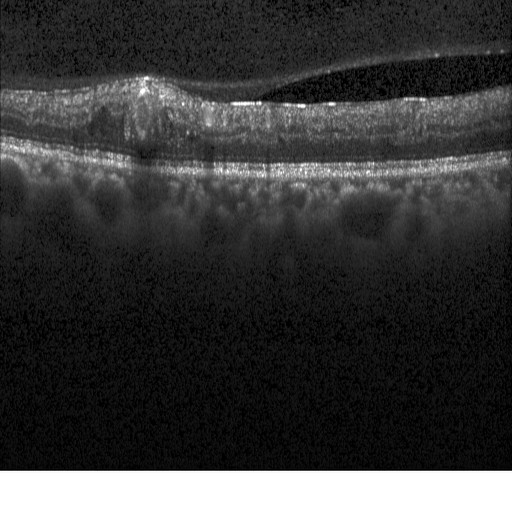

Heidelberg Spectralis OCT system; spectral-domain optical coherence tomography; optical coherence tomography scan — This B-scan demonstrates DME.